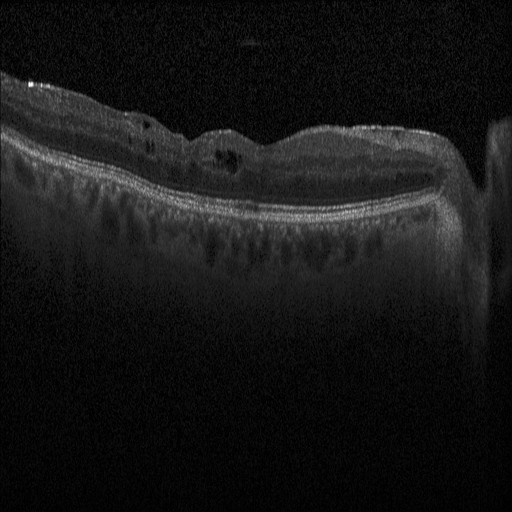
OCT line scan. Centered on the fovea — Impression: diabetic macular edema.